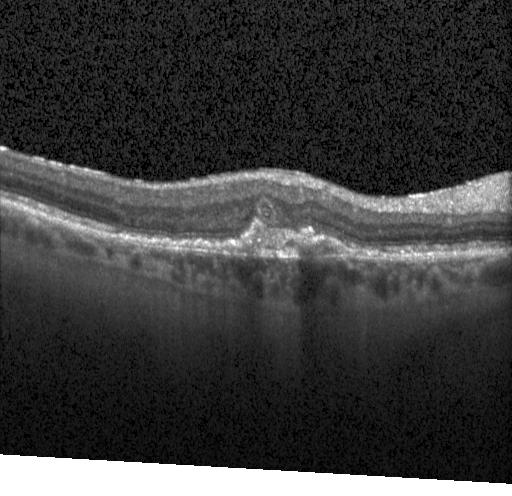 Impression: a choroidal neovascular membrane.